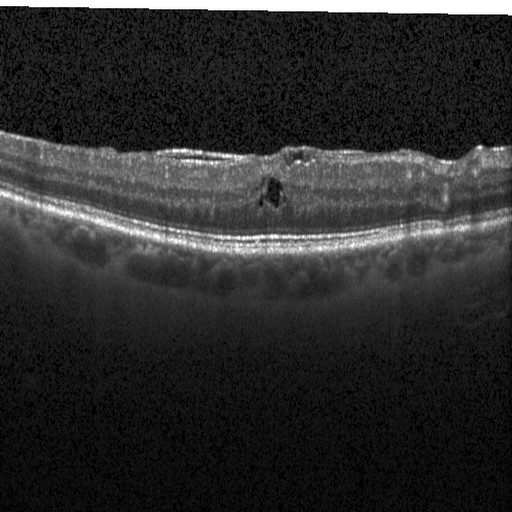

Finding: diabetic macular edema.